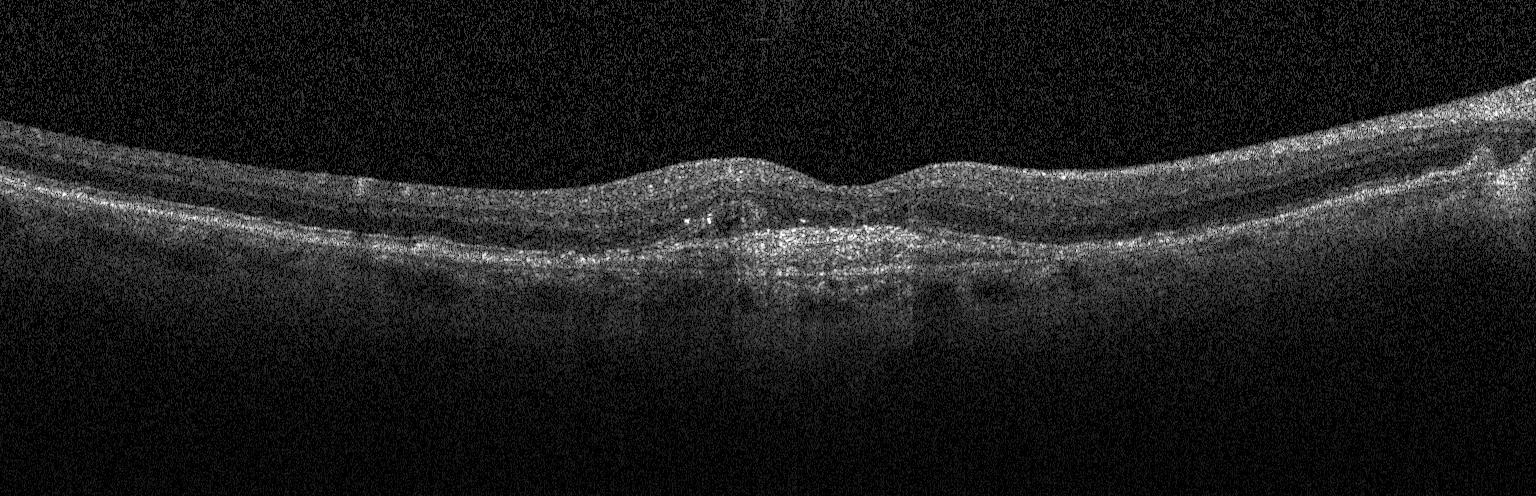
Spectral-domain optical coherence tomography; Heidelberg Spectralis; OCT line scan; centered on the fovea
Finding: a choroidal neovascular membrane.